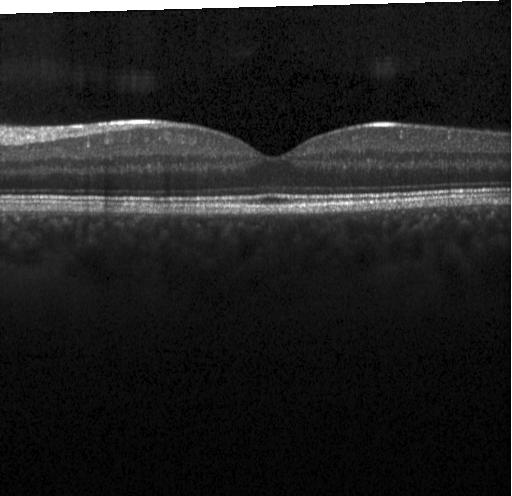 Instrument: Heidelberg Spectralis; optical coherence tomography B-scan; horizontal scan through the fovea. This B-scan demonstrates neither choroidal neovascularization, diabetic macular edema, nor drusen.